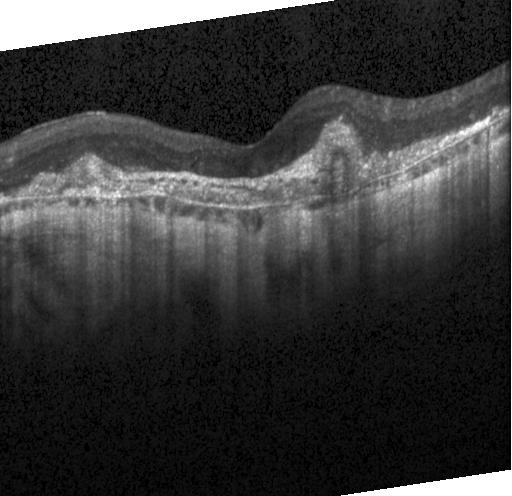
Retinal OCT B-scan, centered on the fovea.
A choroidal neovascular membrane.